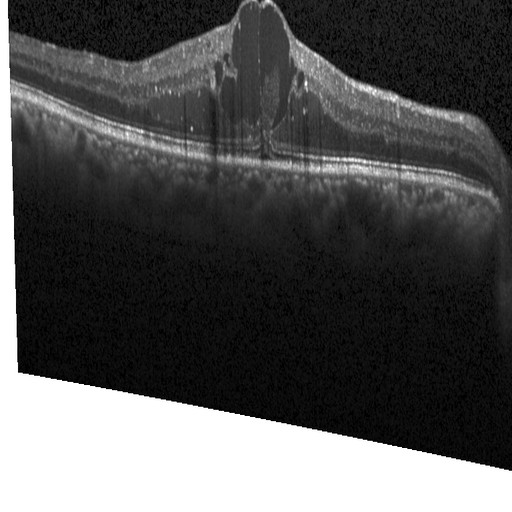 Retinal OCT B-scan — Finding: diabetic macular edema (DME).